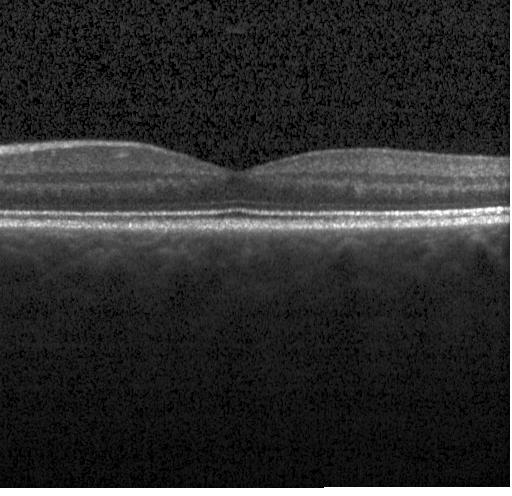

Fovea-centered. OCT line scan.
Macular OCT: neither CNV, DME, nor drusen.